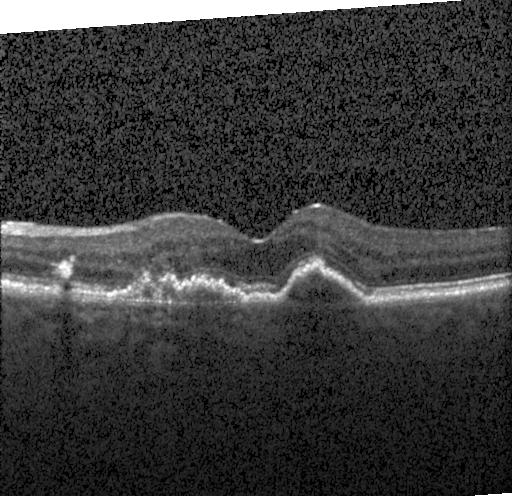
Diagnosis: CNV.